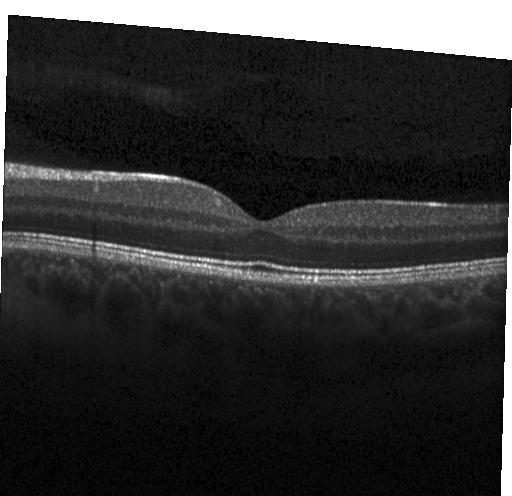

Through the macula. Optical coherence tomography B-scan. Dx: no evidence of choroidal neovascularization, diabetic macular edema, or drusen.